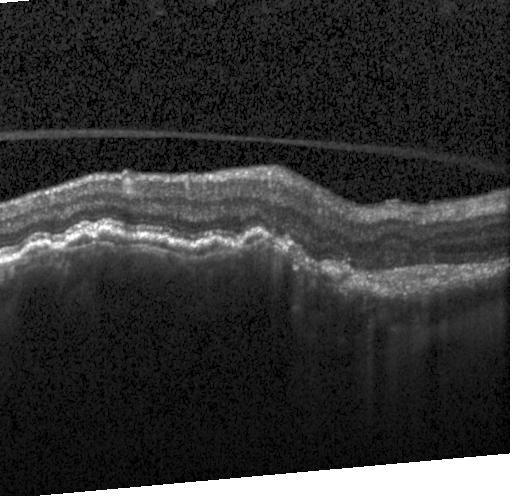
Optical coherence tomography scan; centered on the fovea; Heidelberg Spectralis OCT system; spectral-domain optical coherence tomography.
Impression: CNV.